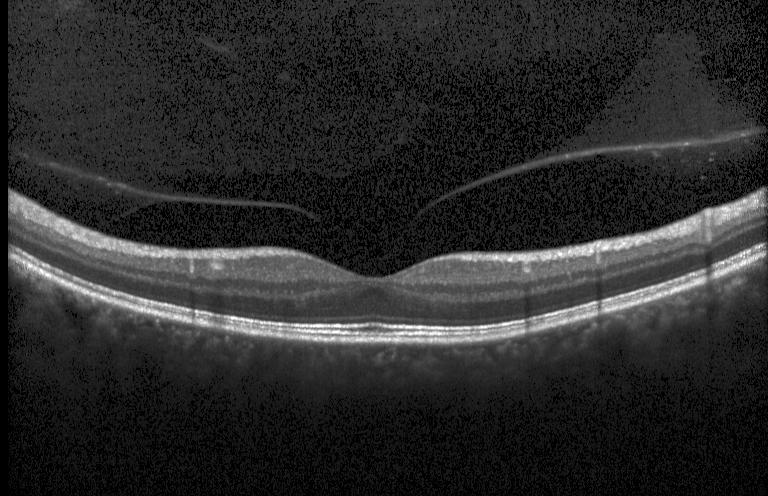

Dx: neither choroidal neovascularization, diabetic macular edema, nor drusen.